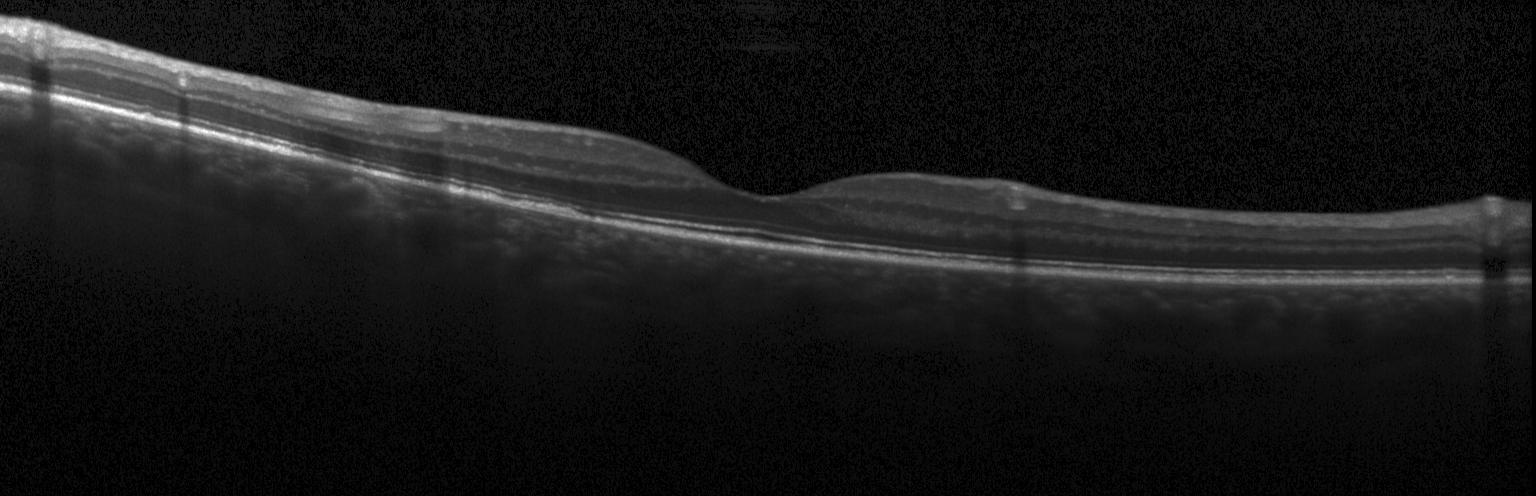

OCT B-scan — This B-scan demonstrates no choroidal neovascularization, no diabetic macular edema, and no drusen.